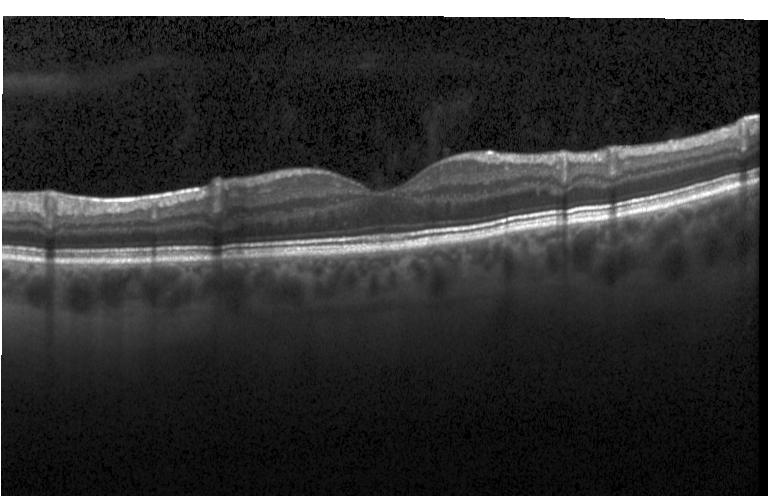
Acquired on a Heidelberg Spectralis · OCT B-scan — Macular OCT: no choroidal neovascularization, diabetic macular edema, or drusen.